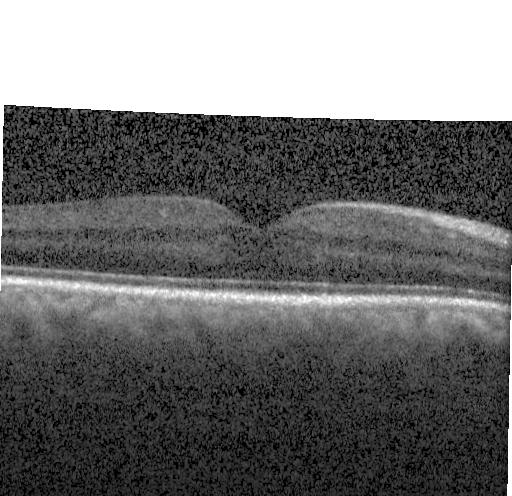 SD-OCT · acquired on a Heidelberg Spectralis · fovea-centered · OCT line scan — Diagnosis: no evidence of CNV, DME, or drusen.